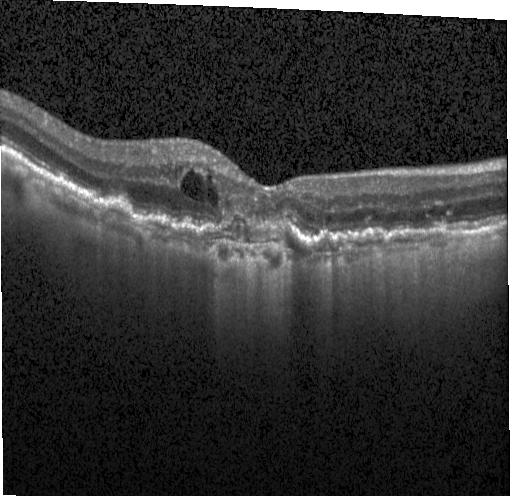 Spectral-domain optical coherence tomography. Fovea-centered. Retinal OCT cross-section.
Diagnosis: choroidal neovascularization (CNV).